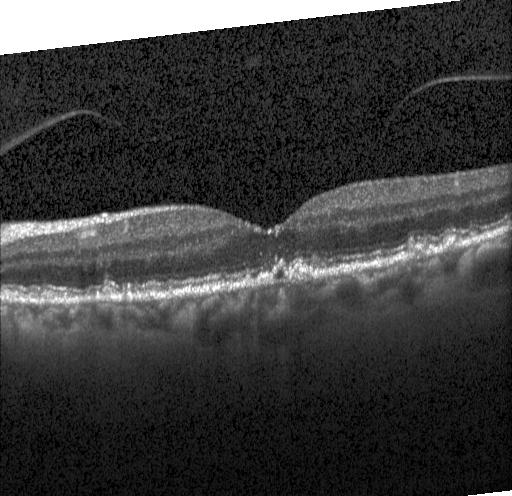
OCT line scan. Macular OCT: sub-RPE drusenoid deposits.